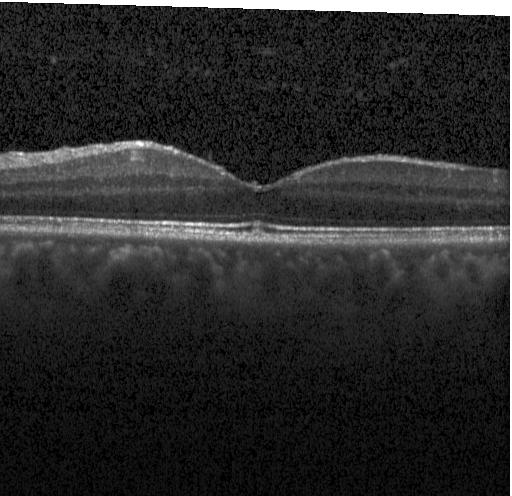

Macular OCT: no evidence of choroidal neovascularization, diabetic macular edema, or drusen.